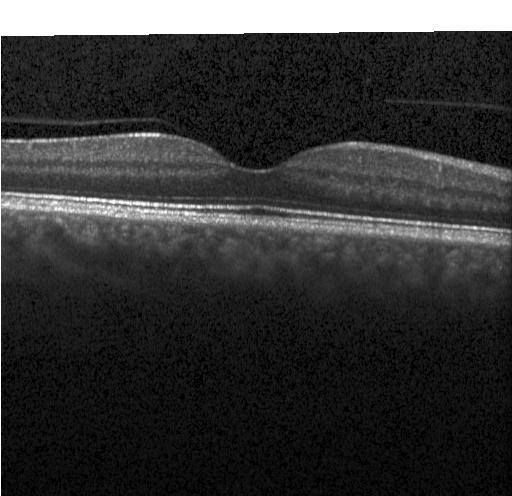

Heidelberg Spectralis OCT system. Spectral-domain OCT. OCT line scan. Macular scan
This B-scan demonstrates no CNV, DME, or drusen.